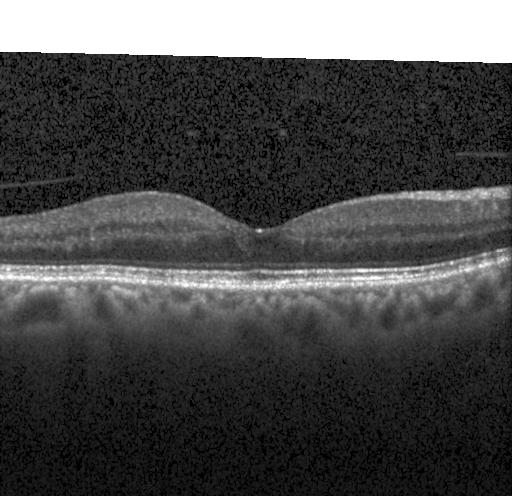 Neither choroidal neovascularization, diabetic macular edema, nor drusen.